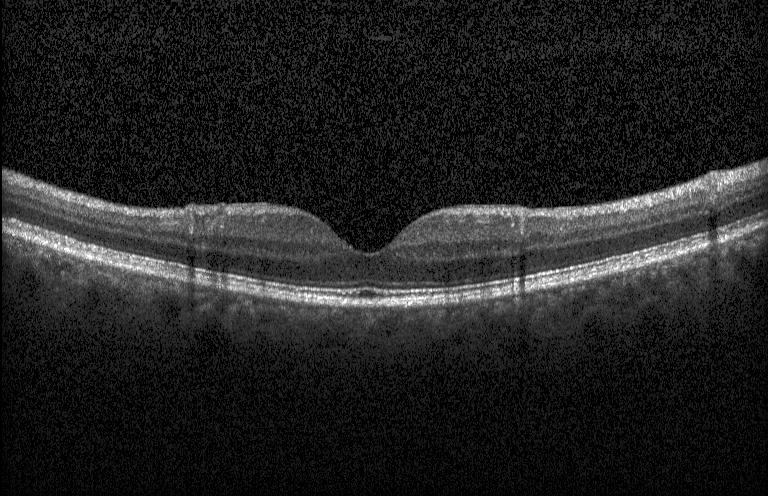

Diagnosis: no choroidal neovascularization, no diabetic macular edema, and no drusen.